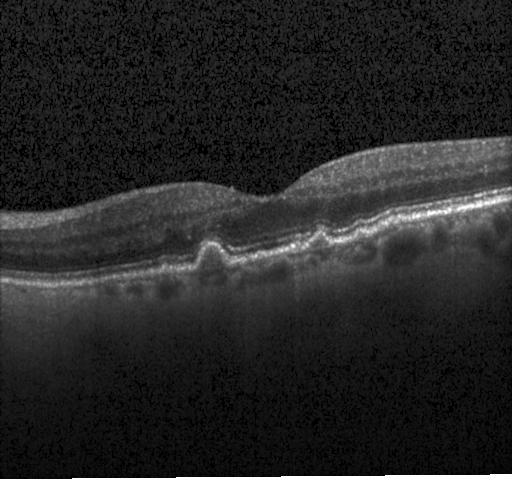

Retinal OCT cross-section; Heidelberg Spectralis; spectral-domain optical coherence tomography.
Finding: multiple drusen.